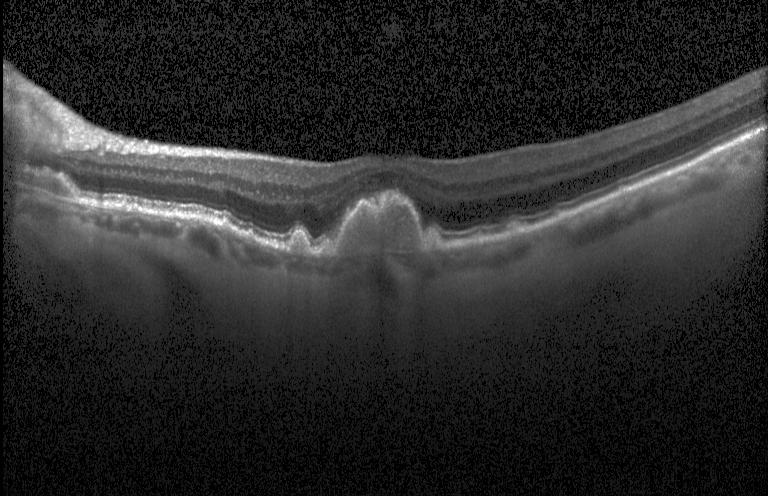 Assessment: drusen.